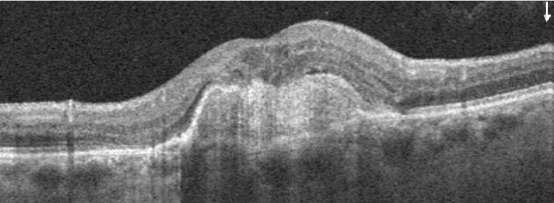

Retinal OCT cross-section
Impression: AMD.